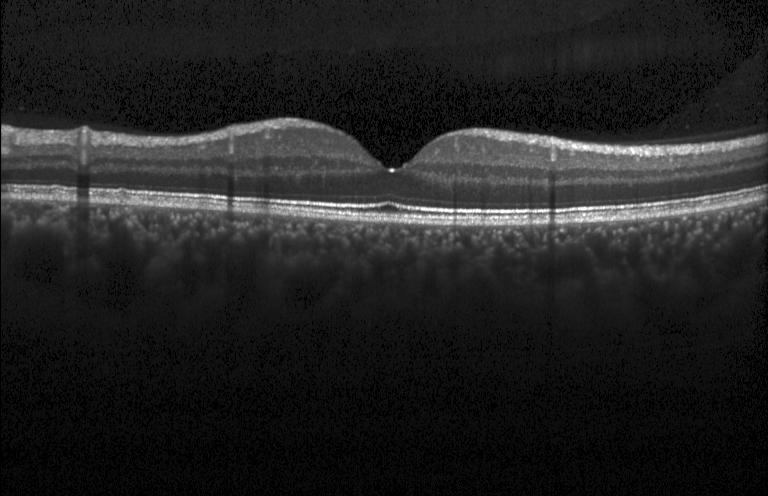 OCT line scan.
Assessment: neither choroidal neovascularization, diabetic macular edema, nor drusen.